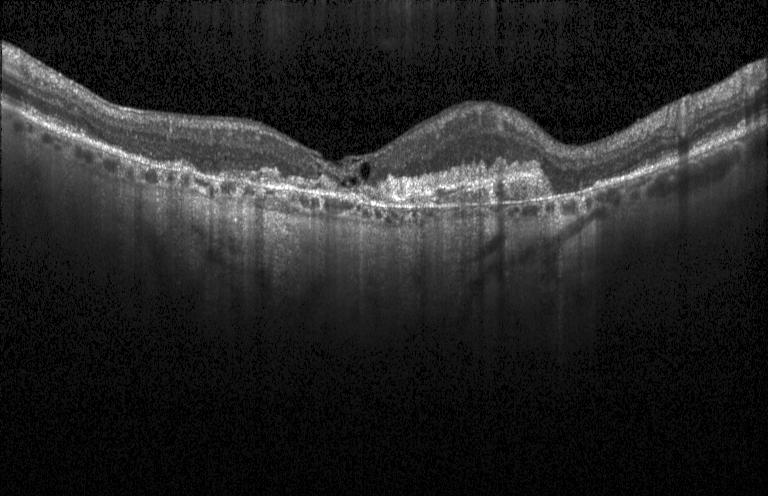 Macular OCT demonstrating a choroidal neovascular membrane.